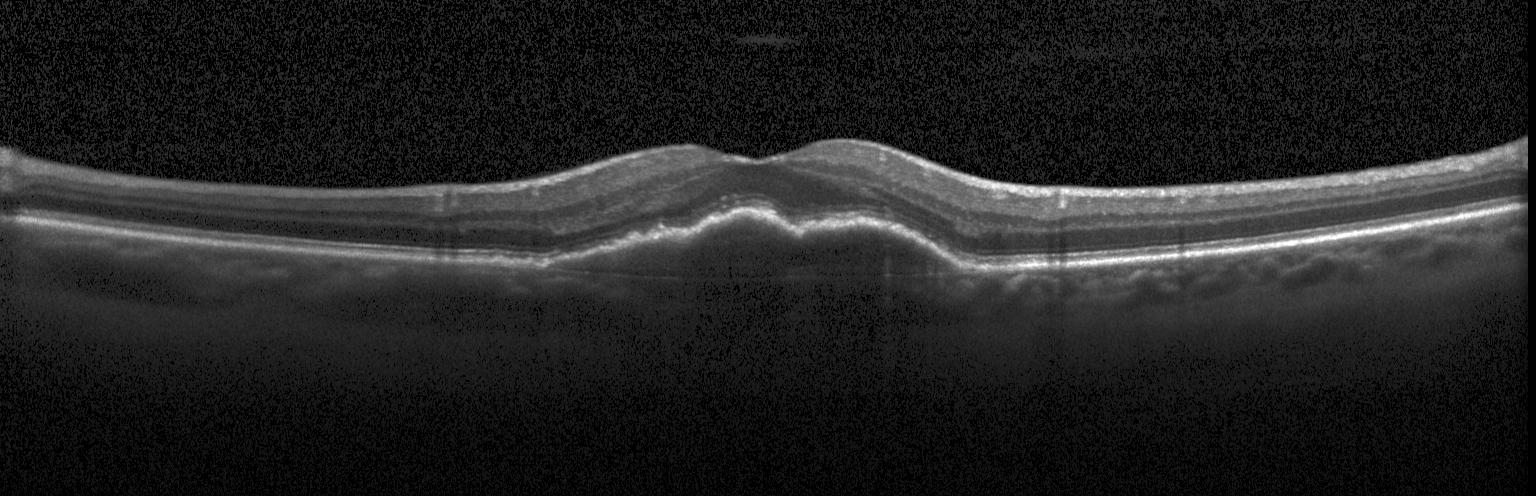

Through the macula · optical coherence tomography B-scan · Heidelberg Spectralis OCT system.
Impression: choroidal neovascularization (CNV).